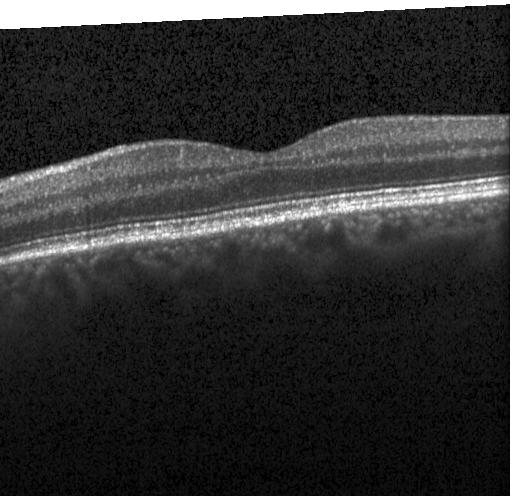 Macular OCT: no choroidal neovascularization, no diabetic macular edema, and no drusen.